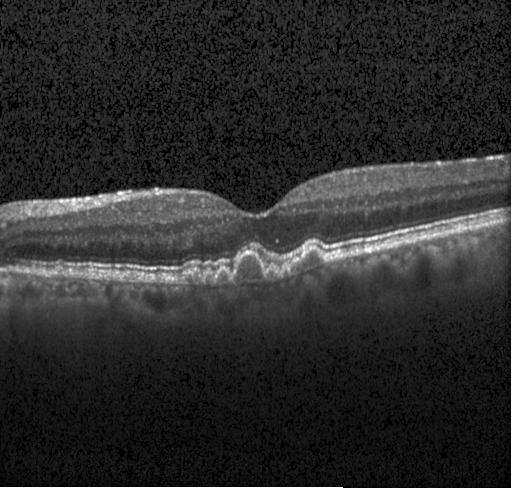
Retinal OCT cross-section
Finding: sub-RPE drusenoid deposits.